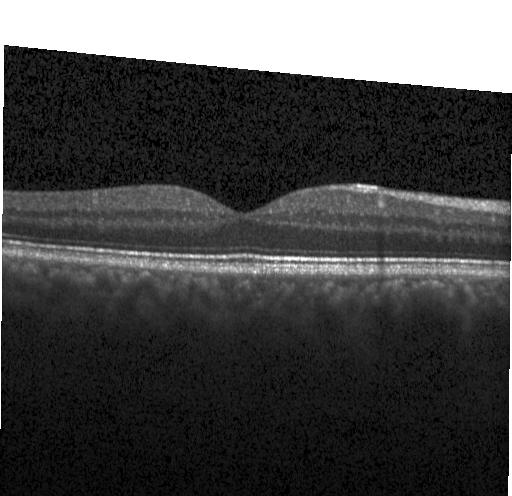
Optical coherence tomography scan, instrument: Heidelberg Spectralis
No CNV, DME, or drusen.